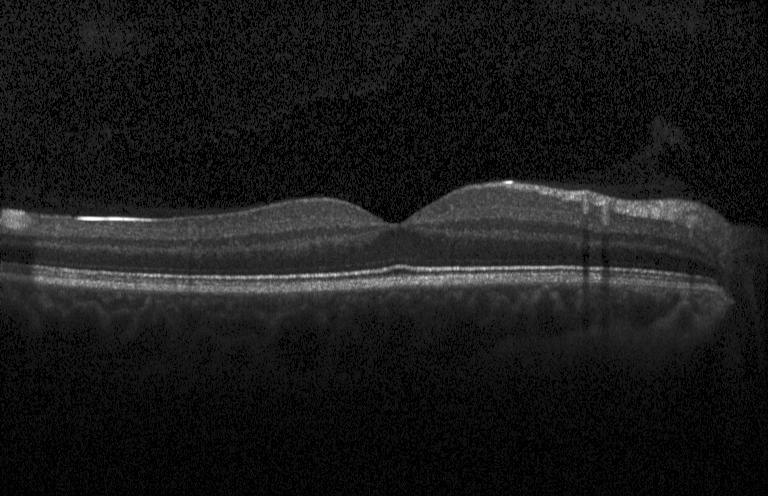

Macular OCT: neither CNV, DME, nor drusen.